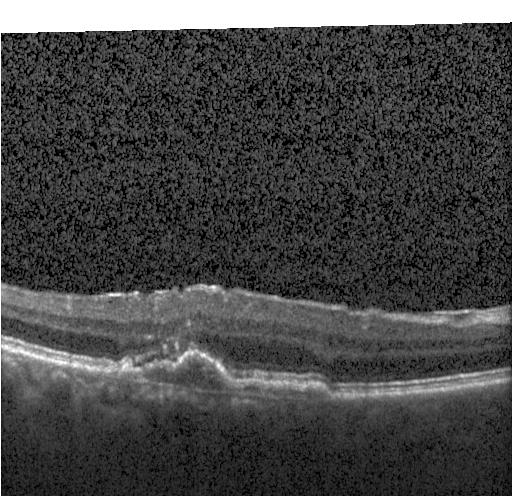 Retinal OCT B-scan, macular scan, Heidelberg Spectralis, spectral-domain OCT.
CNV.